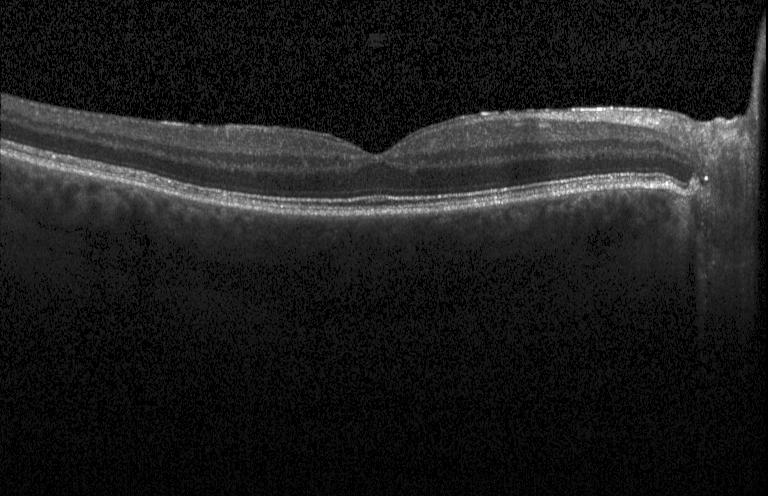
Retinal OCT B-scan.
Assessment: neither choroidal neovascularization, diabetic macular edema, nor drusen.